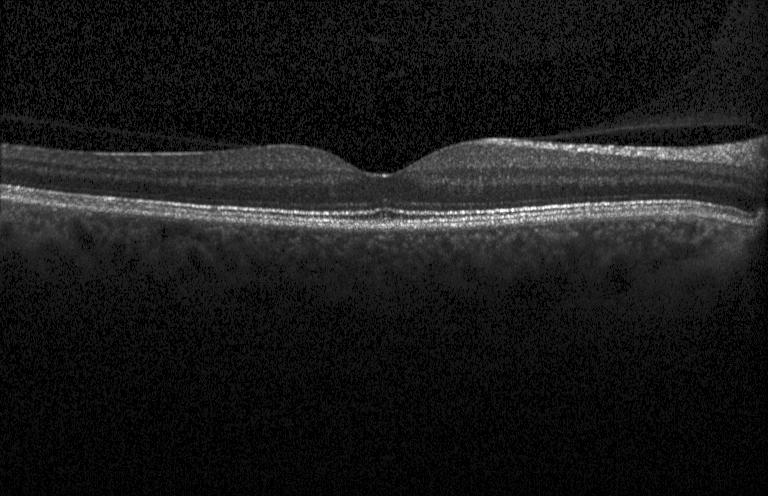
Diagnosis: neither CNV, DME, nor drusen.